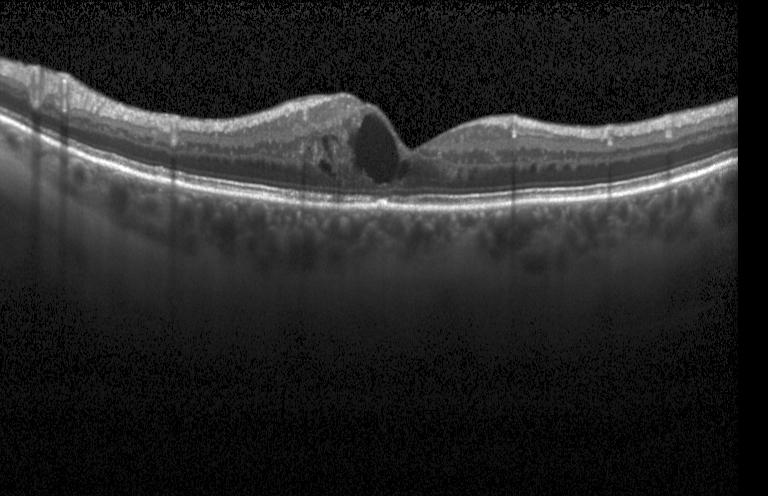 Optical coherence tomography B-scan · centered on the fovea — Diagnosis: DME.